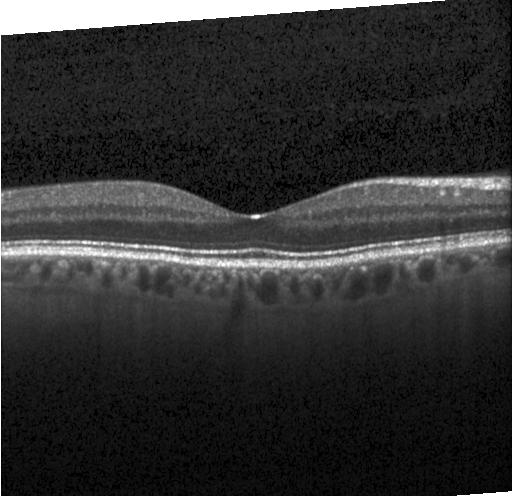

Spectral-domain optical coherence tomography. Optical coherence tomography scan.
Impression: neither choroidal neovascularization, diabetic macular edema, nor drusen.